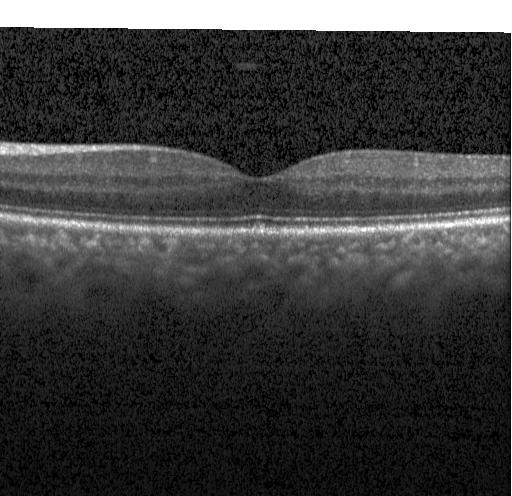 Optical coherence tomography scan; horizontal scan through the fovea; SD-OCT. The scan shows no CNV, DME, or drusen.